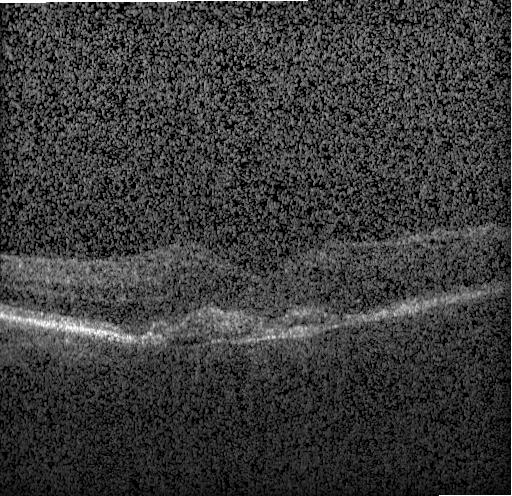
Diagnosis: a choroidal neovascular membrane.